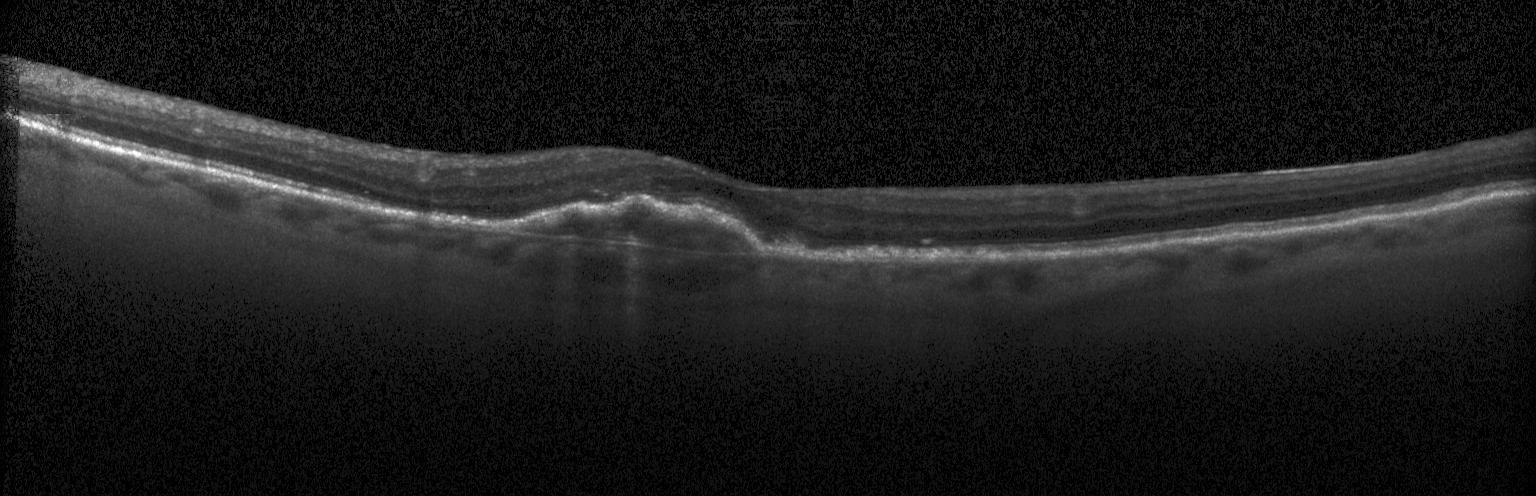

Optical coherence tomography scan · fovea-centered · Heidelberg Spectralis · spectral-domain optical coherence tomography
Impression: a choroidal neovascular membrane.